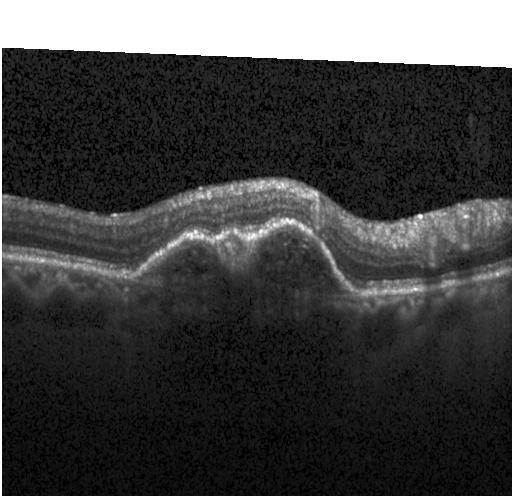 OCT scan showing choroidal neovascularization (CNV).